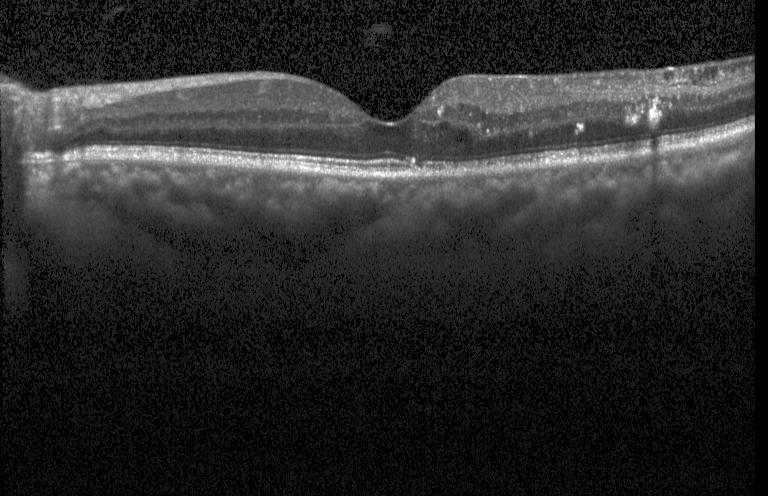

OCT B-scan.
This B-scan demonstrates diabetic macular edema.